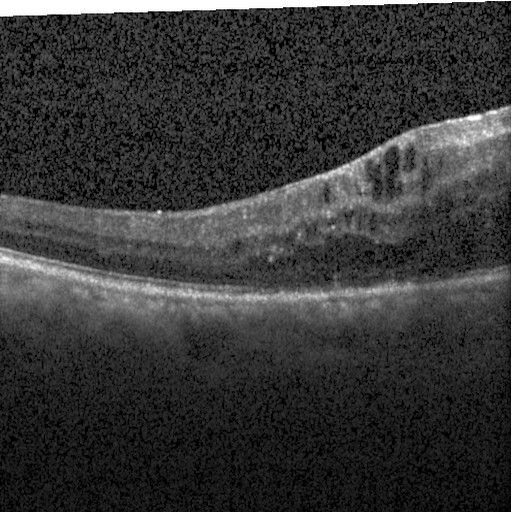 Optical coherence tomography scan.
Finding: diabetic macular edema (DME).